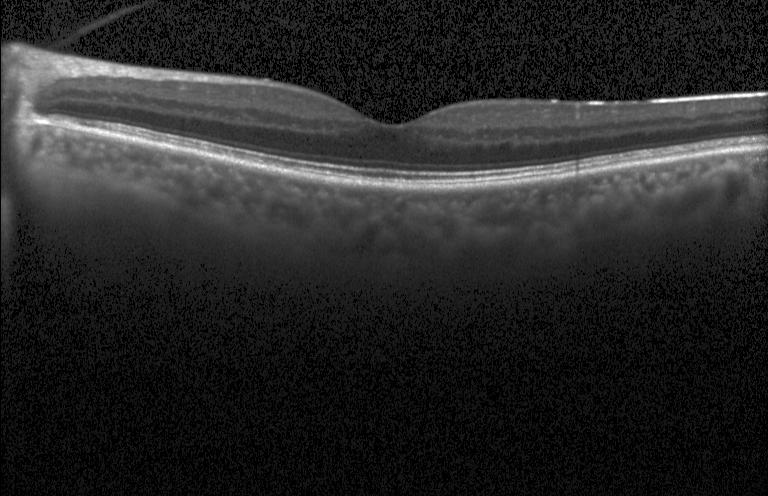
Impression: no choroidal neovascularization, no diabetic macular edema, and no drusen.